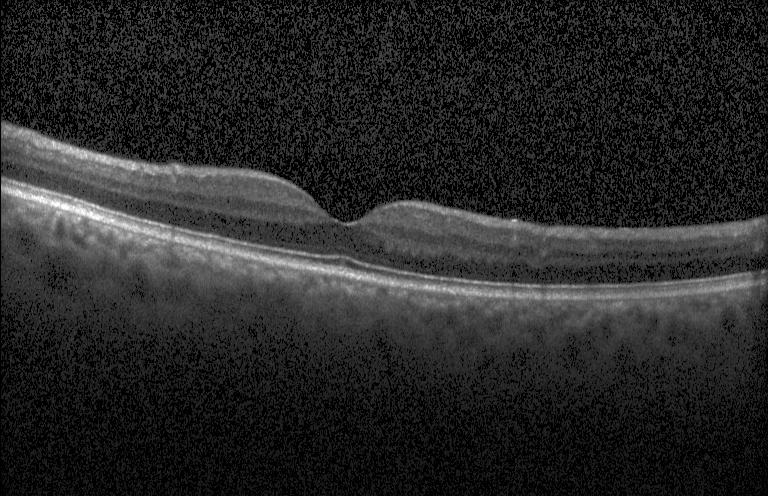
Retinal OCT B-scan; macular scan; acquired on a Heidelberg Spectralis — Finding: neither choroidal neovascularization, diabetic macular edema, nor drusen.